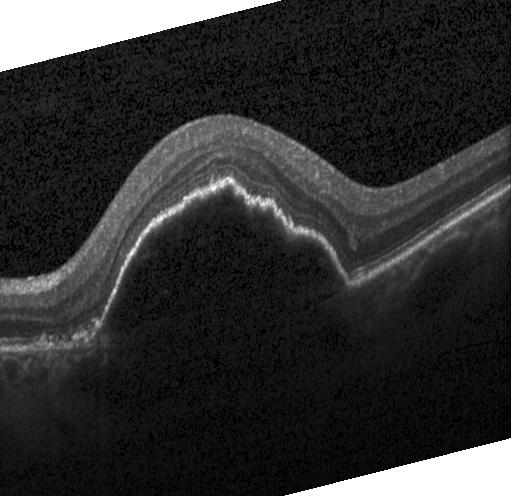 OCT B-scan; Heidelberg Spectralis; SD-OCT; centered on the fovea
Impression: CNV.